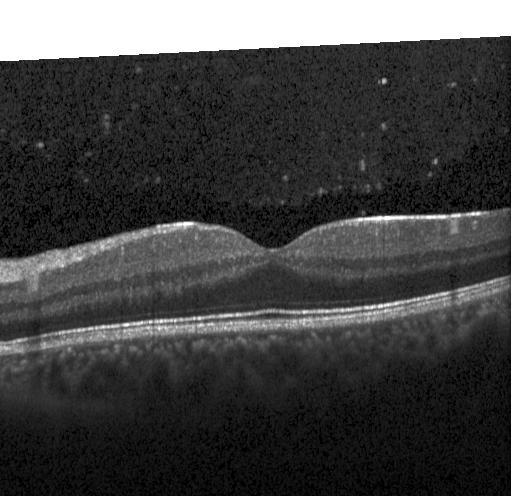
OCT line scan, through the macula — Dx: no CNV, no DME, and no drusen.